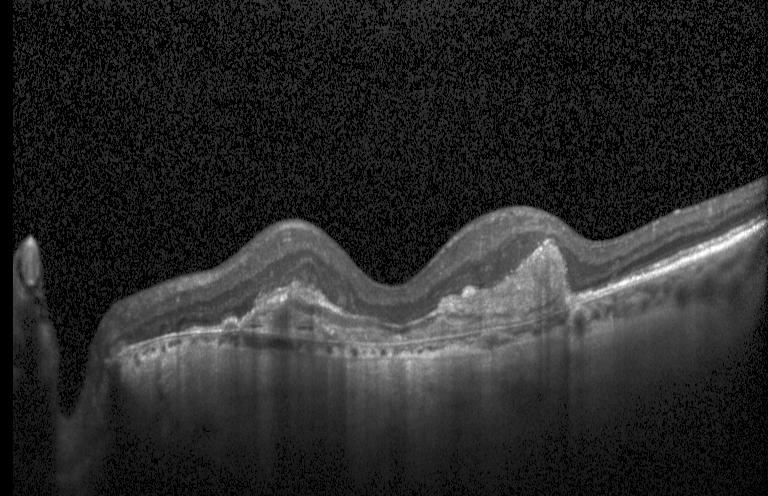
Impression: a choroidal neovascular membrane.